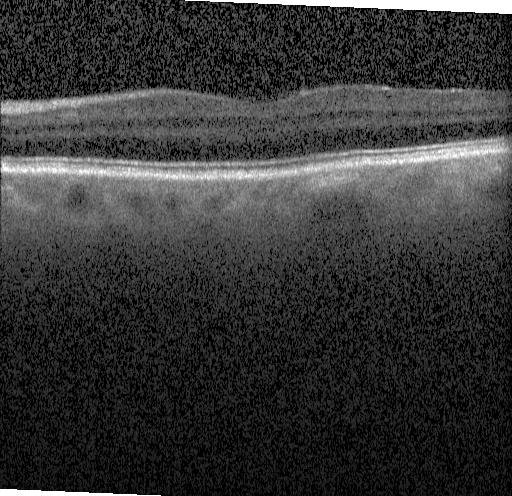

Heidelberg Spectralis; centered on the fovea; OCT B-scan; spectral-domain optical coherence tomography. Diagnosis: no choroidal neovascularization, diabetic macular edema, or drusen.